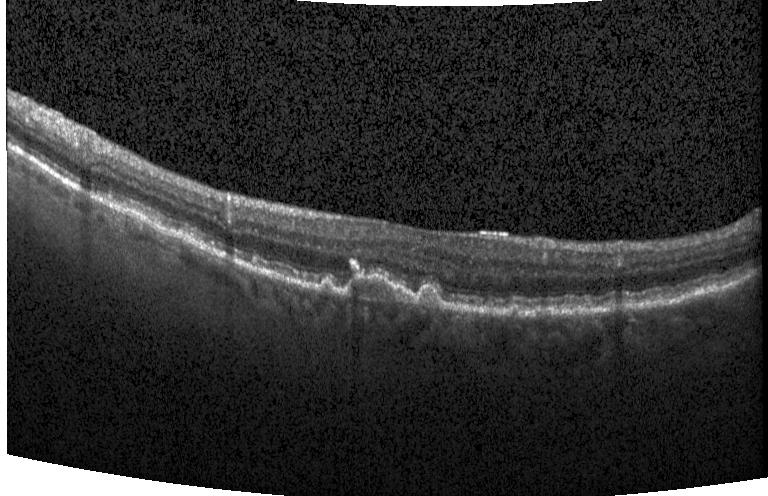 Heidelberg Spectralis OCT system. Optical coherence tomography scan. Spectral-domain optical coherence tomography. Dx: a choroidal neovascular membrane.